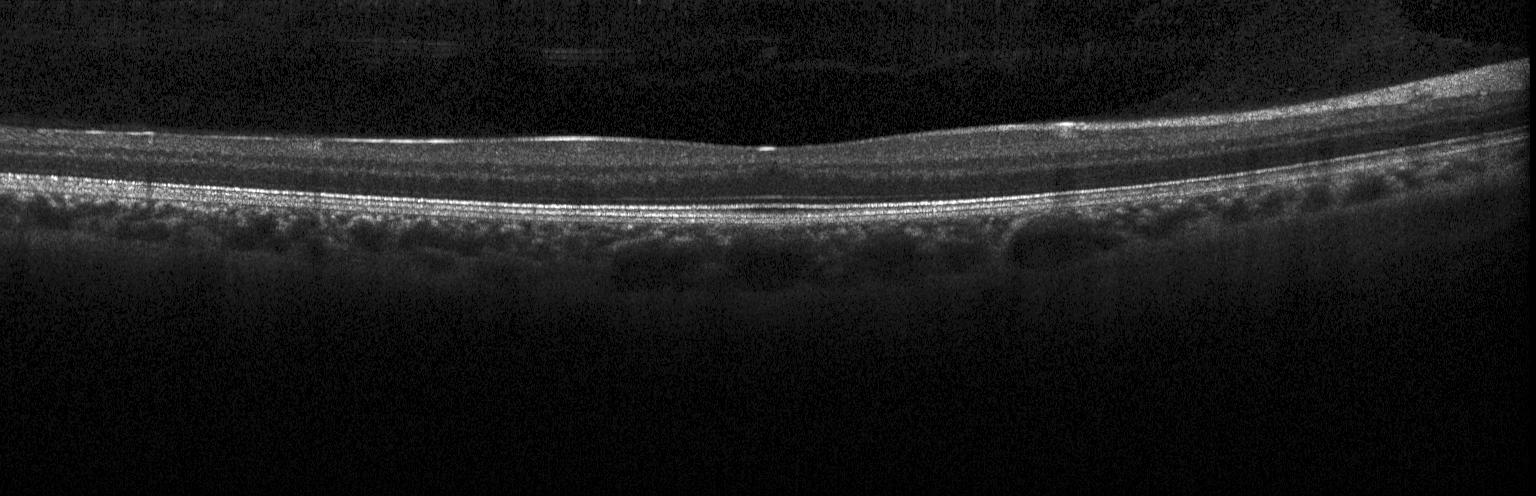

OCT line scan · Heidelberg Spectralis OCT system.
No CNV, DME, or drusen.